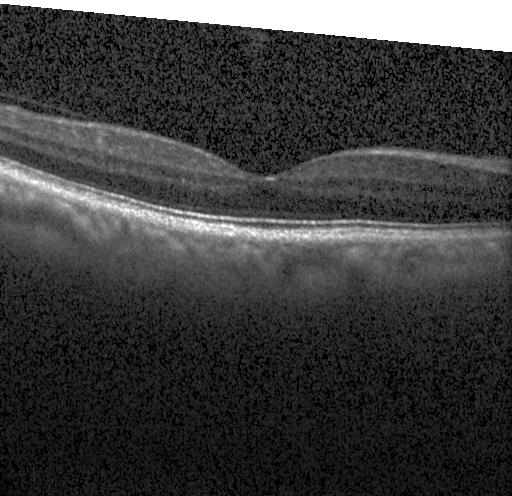
Heidelberg Spectralis OCT system, retinal OCT cross-section, centered on the fovea — Dx: neither CNV, DME, nor drusen.